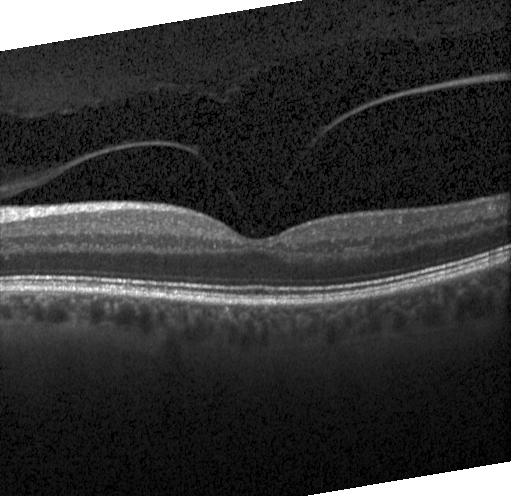 Impression: no CNV, no DME, and no drusen.